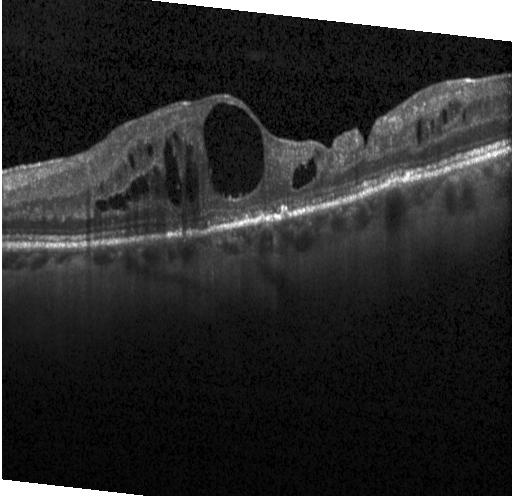

Optical coherence tomography B-scan
The scan shows diabetic macular edema.